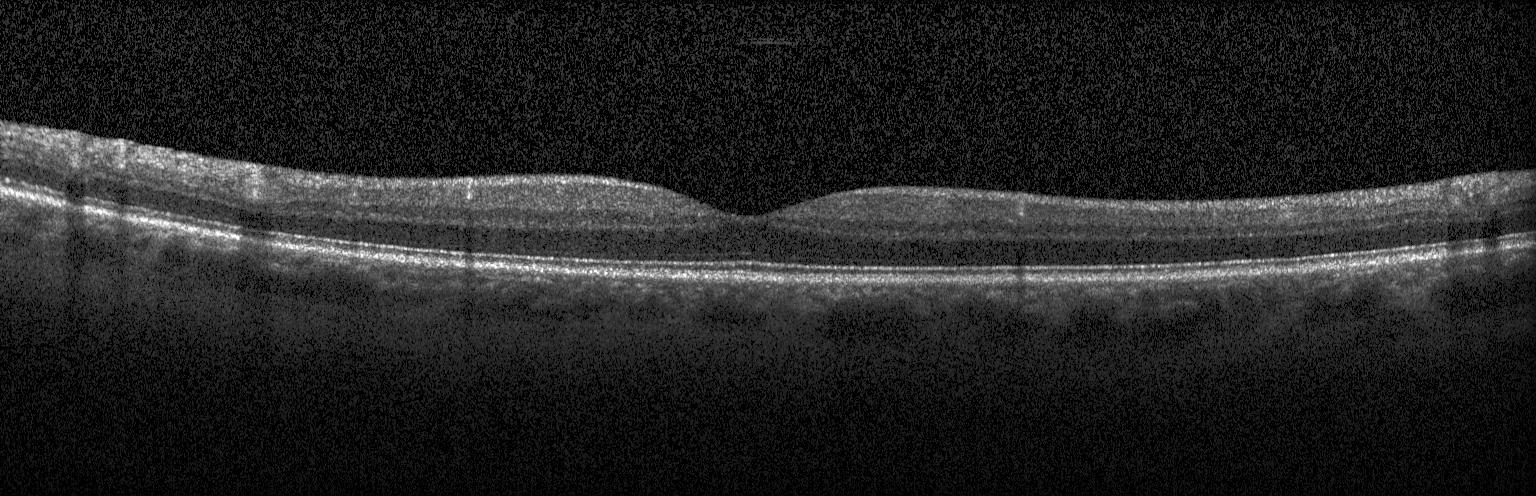 This B-scan demonstrates no CNV, DME, or drusen.